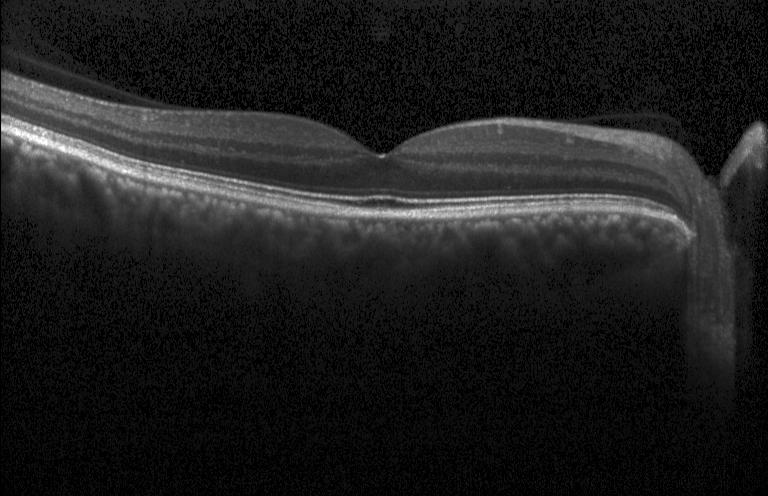
Spectral-domain OCT B-scan: no evidence of choroidal neovascularization, diabetic macular edema, or drusen.